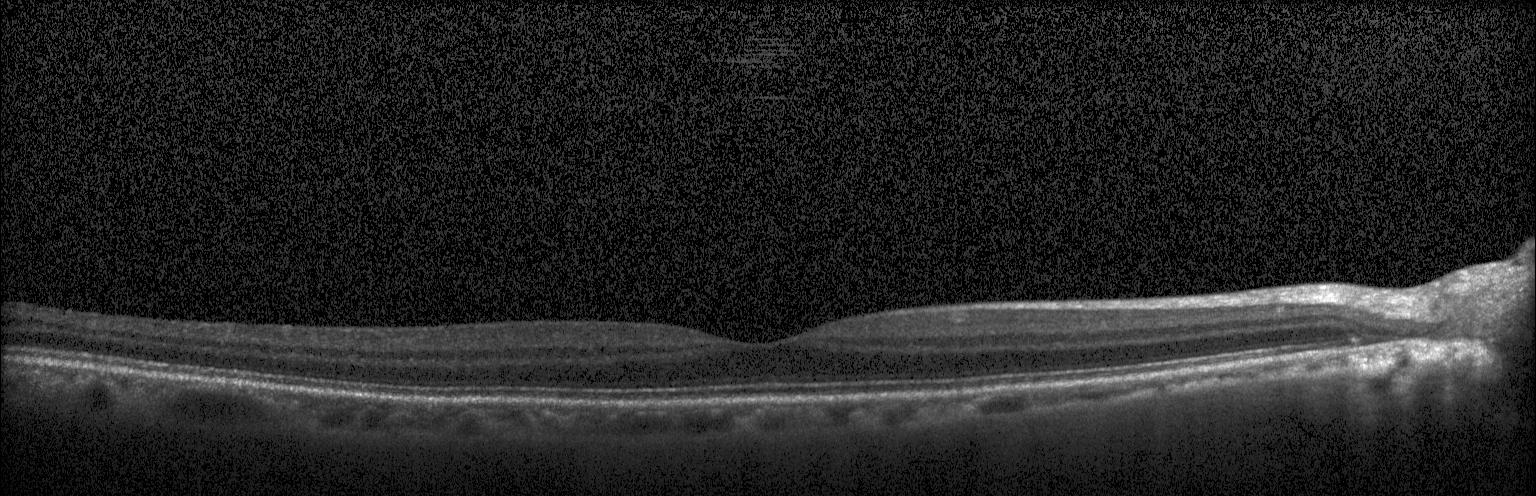 Retinal OCT cross-section showing no choroidal neovascularization, no diabetic macular edema, and no drusen.